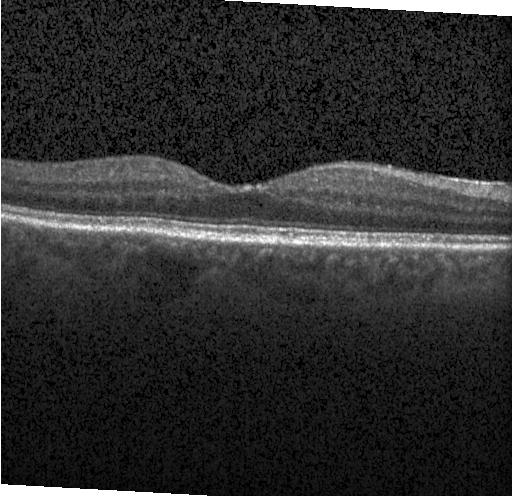
OCT B-scan. Spectral-domain optical coherence tomography. Heidelberg Spectralis OCT system. Fovea-centered.
Diagnosis: neither choroidal neovascularization, diabetic macular edema, nor drusen.